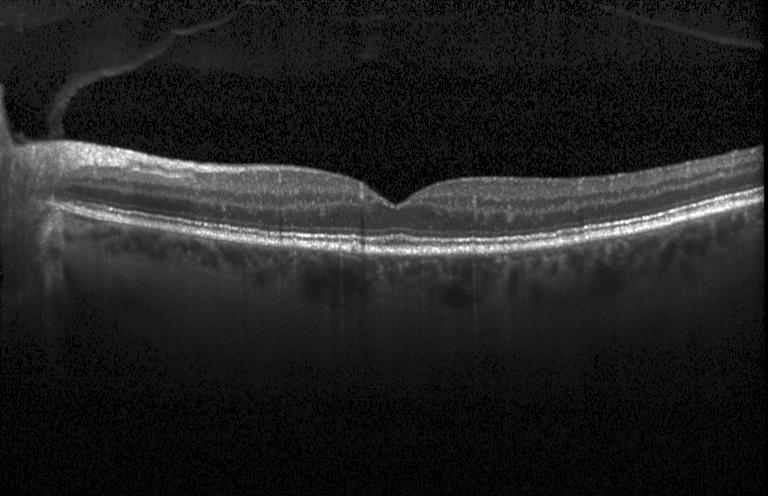
Diagnosis: no choroidal neovascularization, no diabetic macular edema, and no drusen.